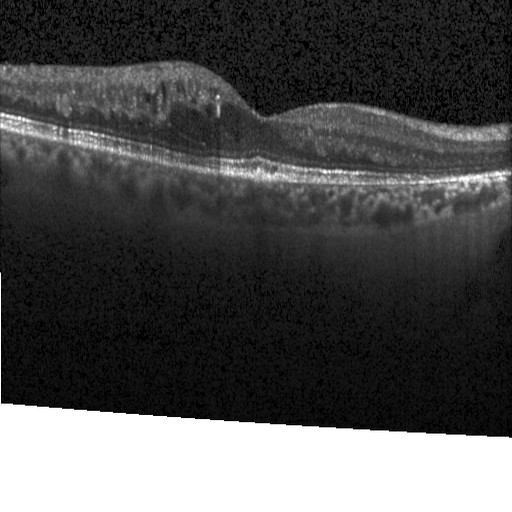
Retinal OCT B-scan · Heidelberg Spectralis · horizontal scan through the fovea · spectral-domain optical coherence tomography.
Macular OCT: diabetic macular edema (DME).